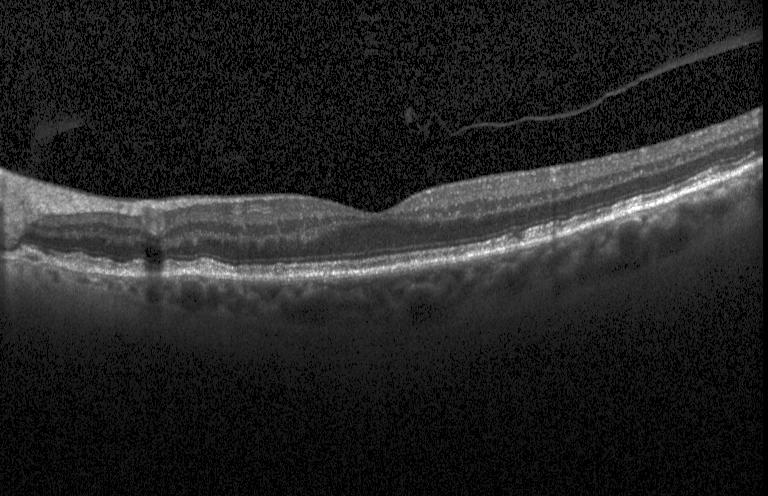
Diagnosis: sub-RPE drusenoid deposits.